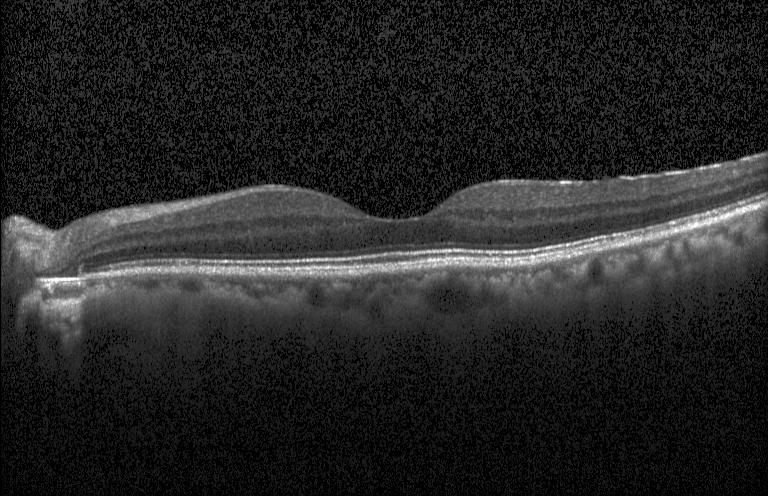
Heidelberg Spectralis OCT system. Centered on the fovea. Retinal OCT B-scan — Finding: no choroidal neovascularization, diabetic macular edema, or drusen.